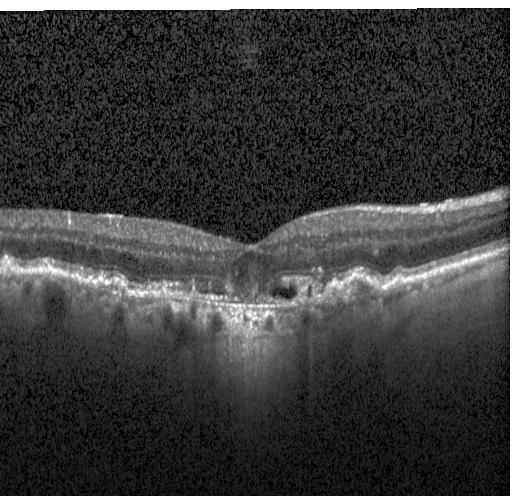
OCT line scan. SD-OCT.
Impression: a choroidal neovascular membrane.